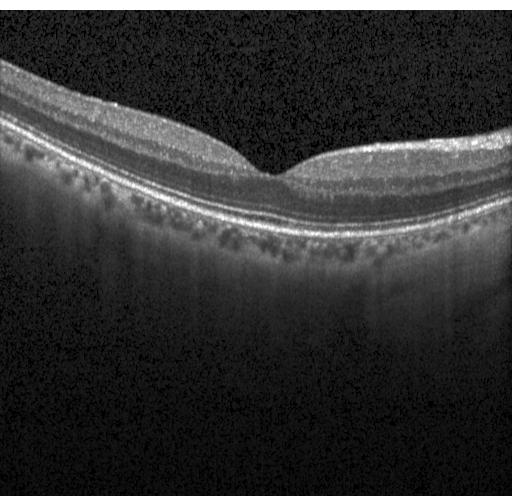
Macular OCT: no CNV, DME, or drusen.